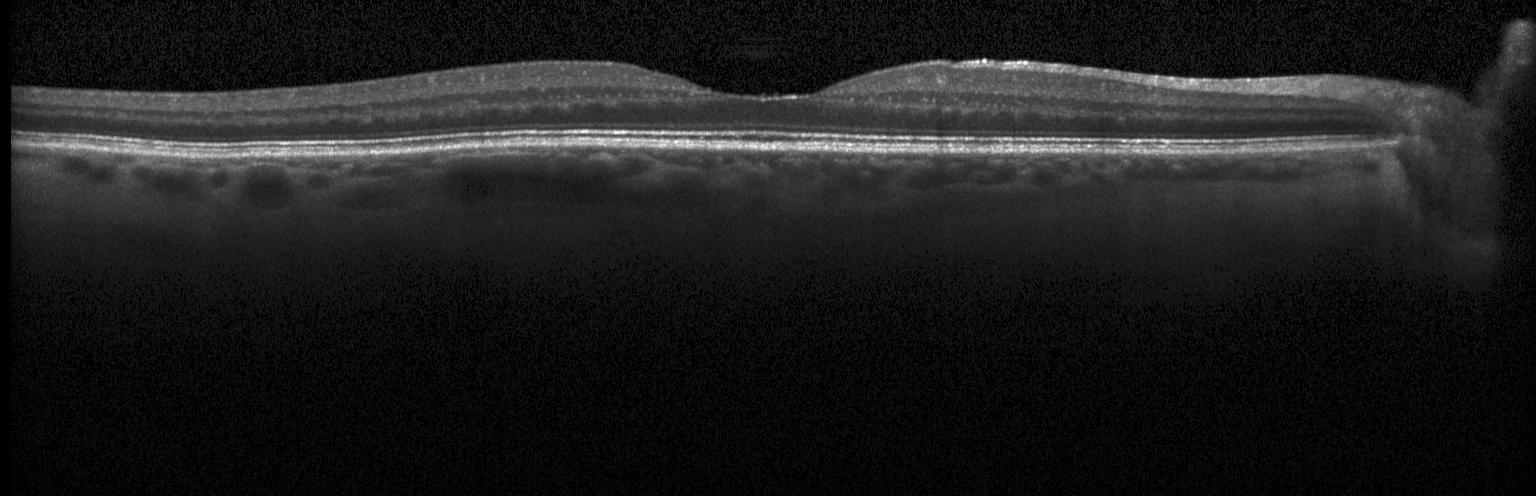

No choroidal neovascularization, diabetic macular edema, or drusen.